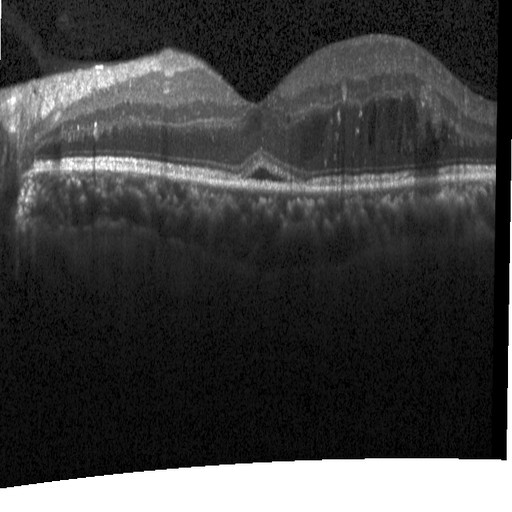

SD-OCT · optical coherence tomography scan · instrument: Heidelberg Spectralis
Macular OCT: DME.